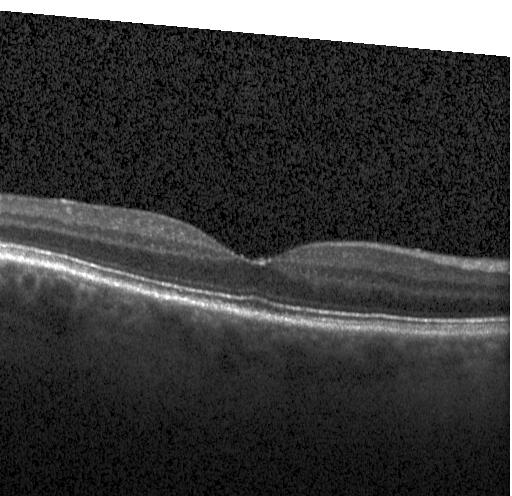

Finding: no choroidal neovascularization, no diabetic macular edema, and no drusen.